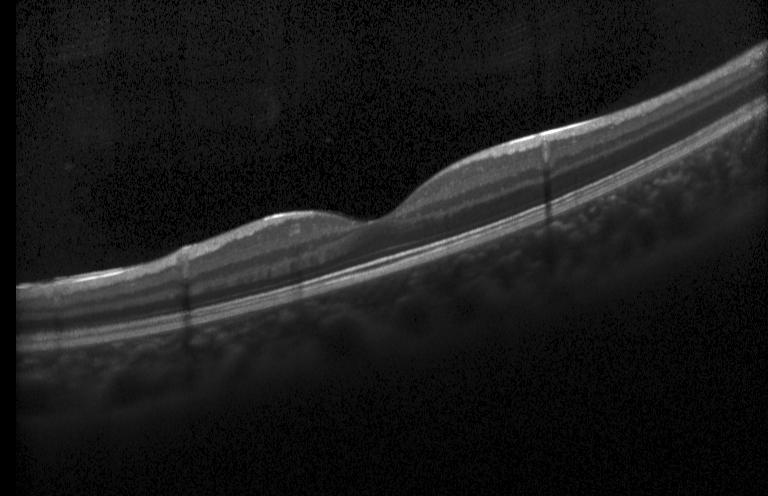

Spectral-domain OCT B-scan: no evidence of CNV, DME, or drusen.